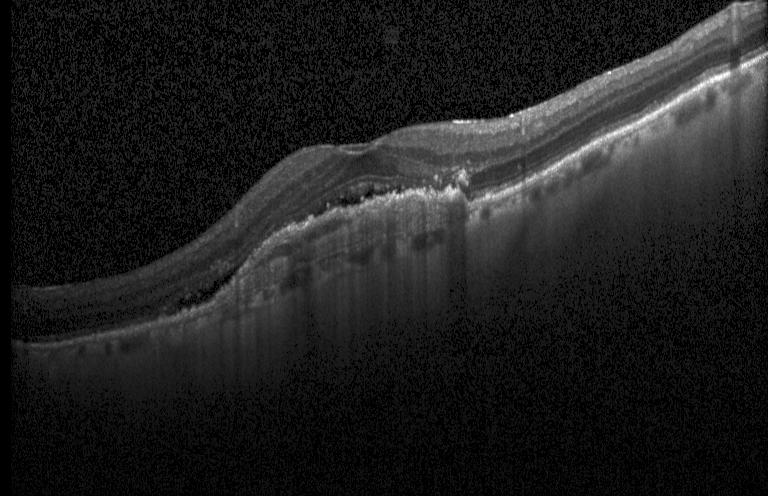
Retinal OCT B-scan. SD-OCT. Through the macula. Acquired on a Heidelberg Spectralis — Diagnosis: CNV.